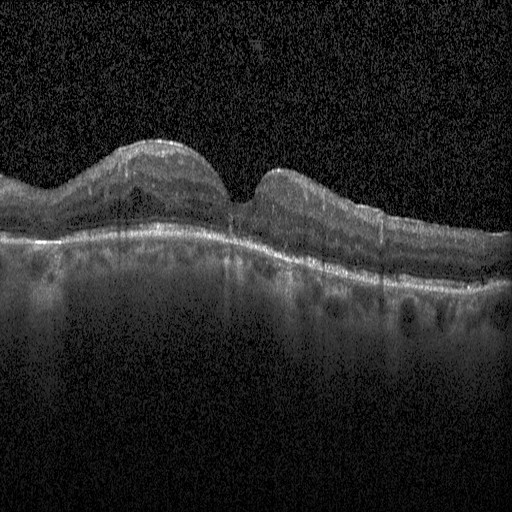
Optical coherence tomography B-scan. Fovea-centered — Diagnosis: diabetic macular edema (DME).